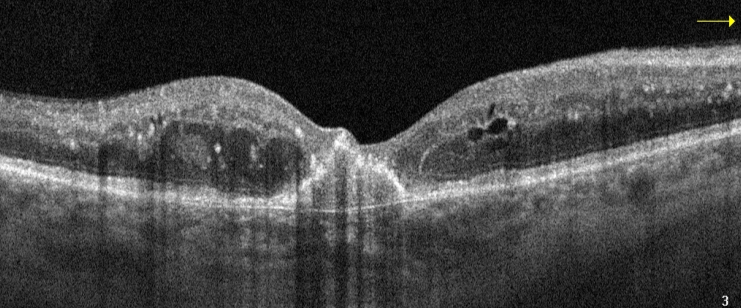
OCT B-scan.
OCT finding: diabetic macular edema.